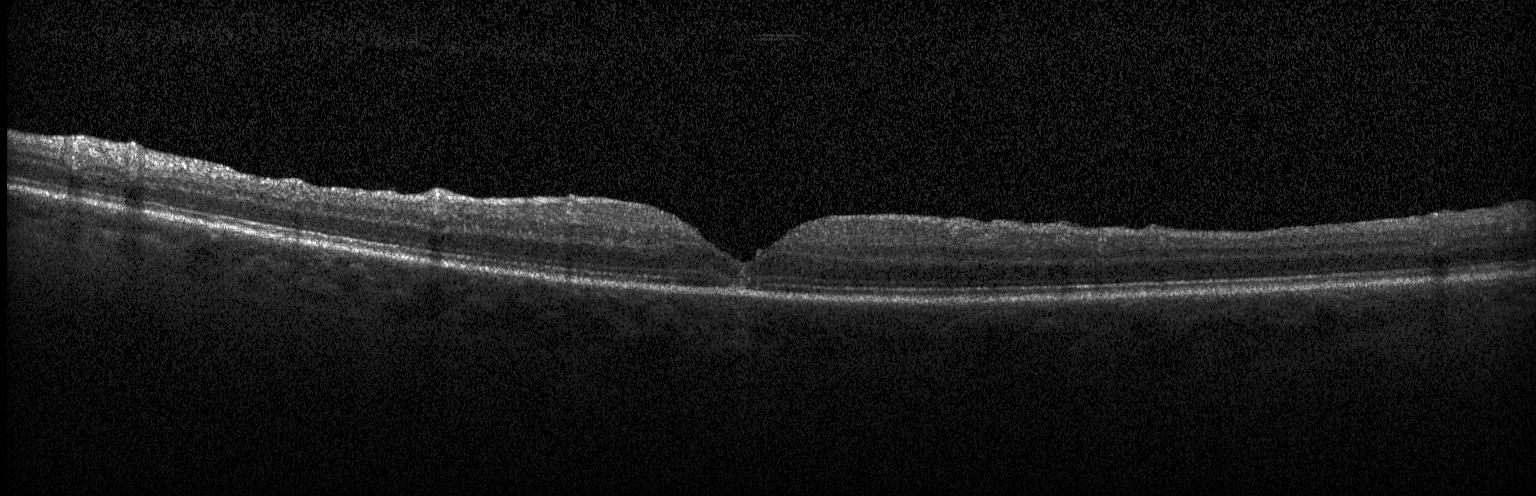
Impression: no evidence of choroidal neovascularization, diabetic macular edema, or drusen.